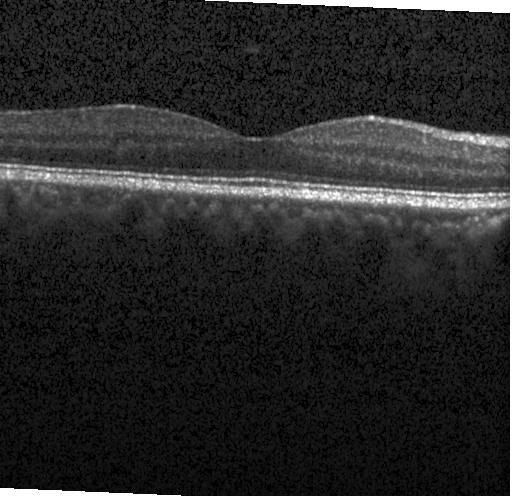 Instrument: Heidelberg Spectralis · optical coherence tomography B-scan.
Macular OCT: no choroidal neovascularization, diabetic macular edema, or drusen.